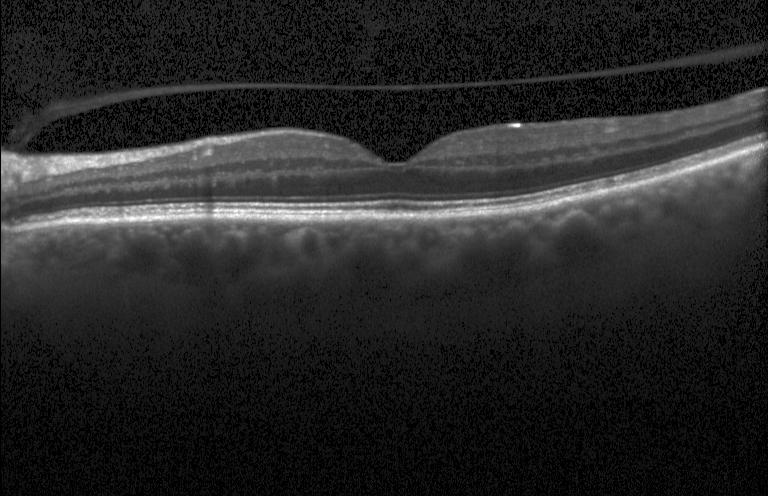

The scan shows no choroidal neovascularization, no diabetic macular edema, and no drusen.